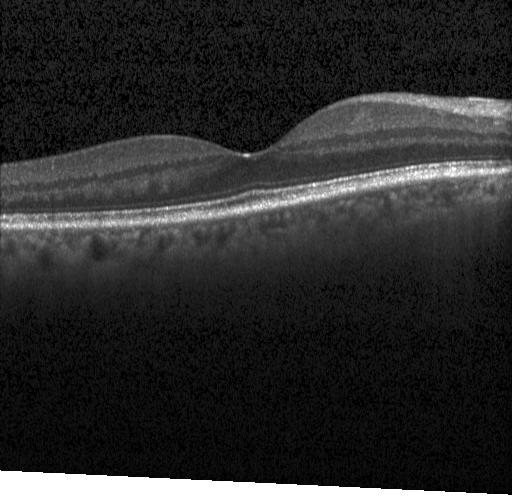
Instrument: Heidelberg Spectralis; spectral-domain OCT; through the macula; OCT B-scan — This B-scan demonstrates no CNV, DME, or drusen.